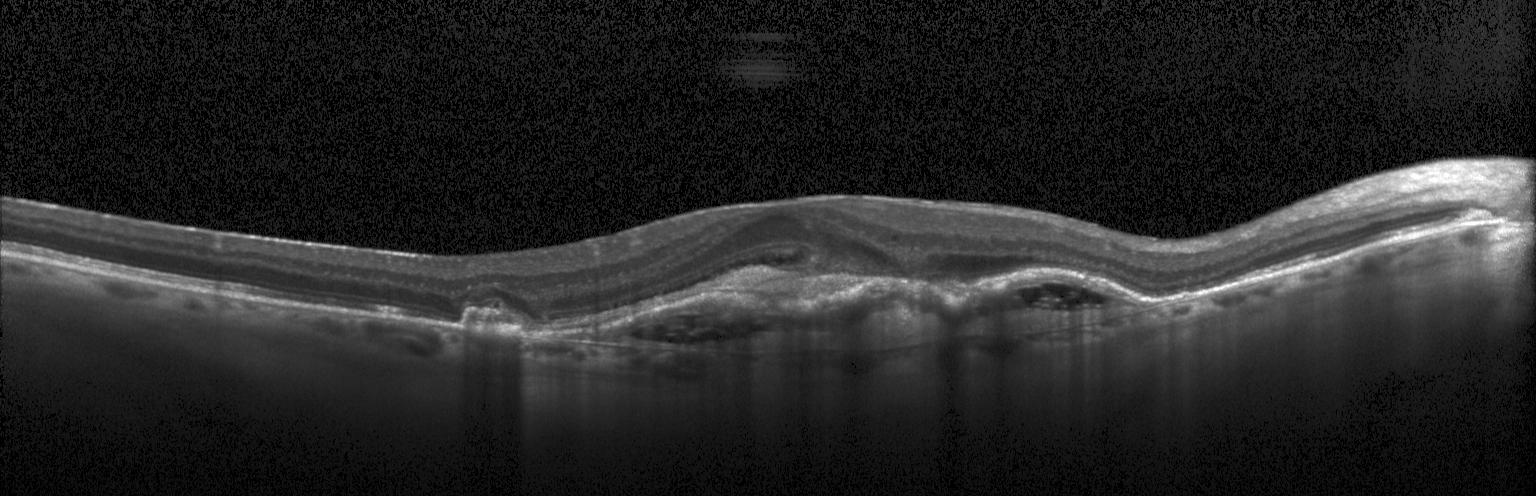
OCT scan showing a choroidal neovascular membrane.